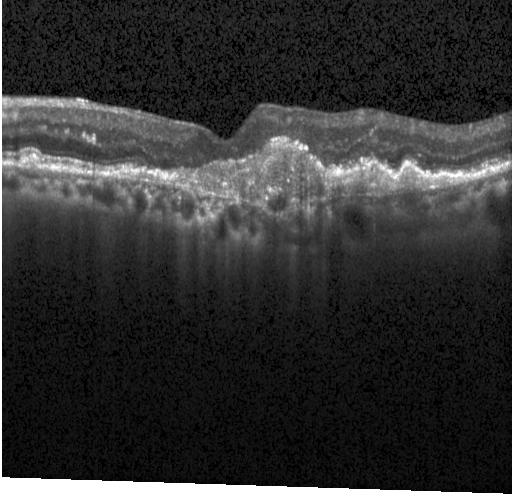
Centered on the fovea; optical coherence tomography scan.
Diagnosis: a choroidal neovascular membrane.